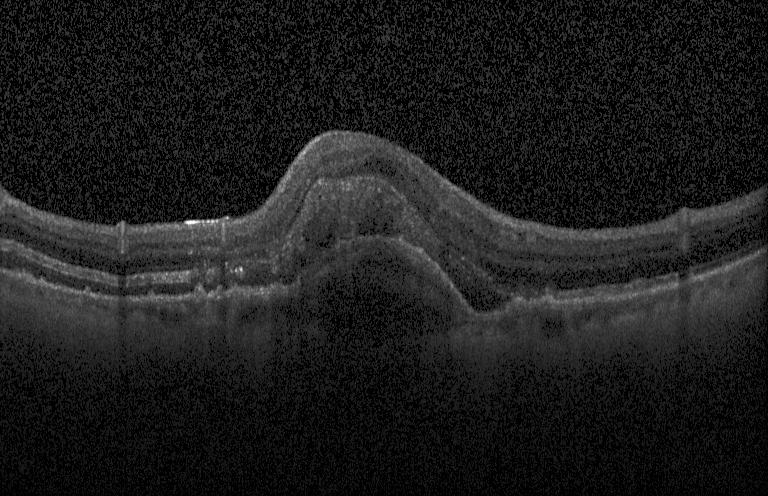 Retinal OCT cross-section.
Impression: a choroidal neovascular membrane.